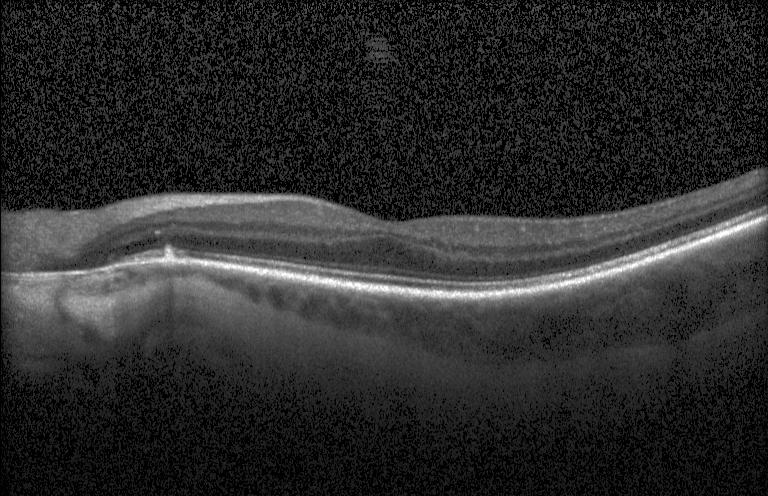

Impression: drusen.